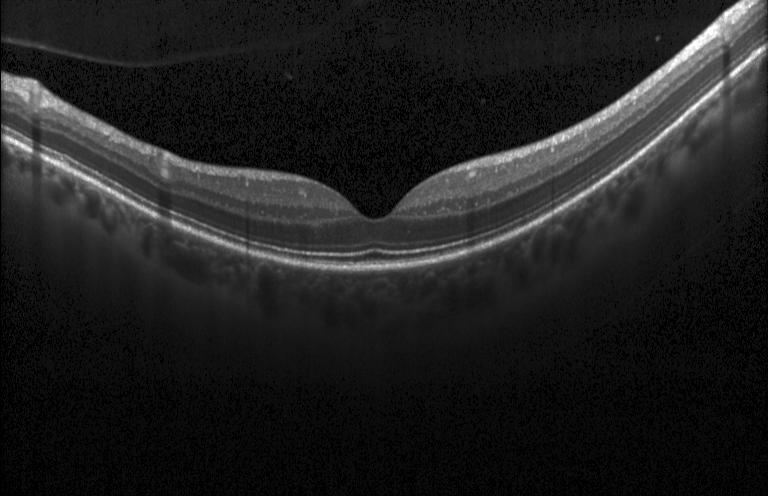 OCT B-scan, Heidelberg Spectralis, spectral-domain optical coherence tomography
The scan shows no CNV, DME, or drusen.